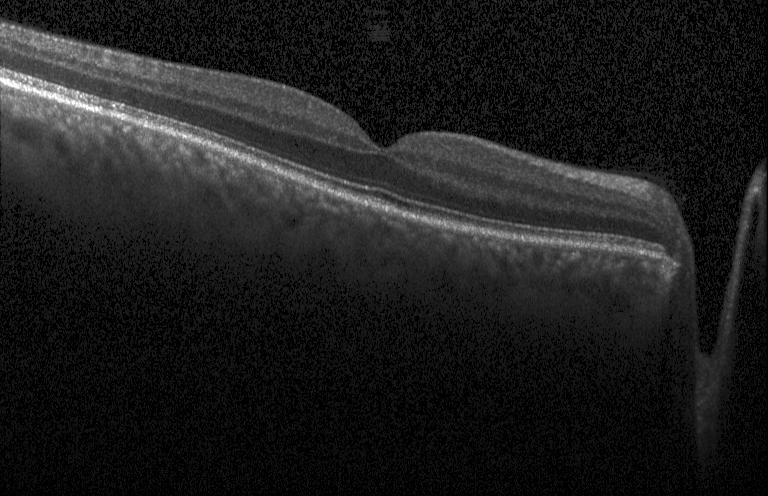 OCT line scan
Assessment: no choroidal neovascularization, no diabetic macular edema, and no drusen.